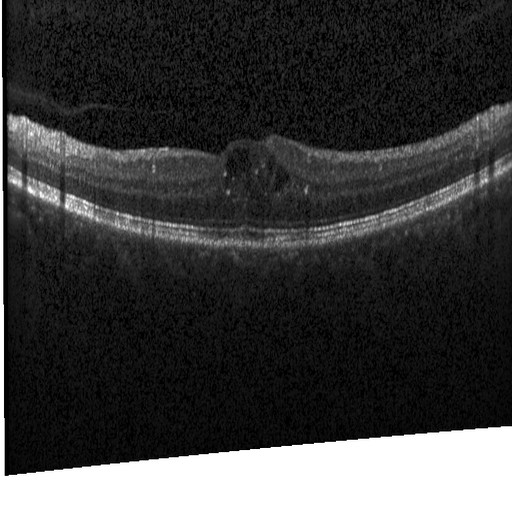
Retinal OCT B-scan, Heidelberg Spectralis — Dx: diabetic macular edema.